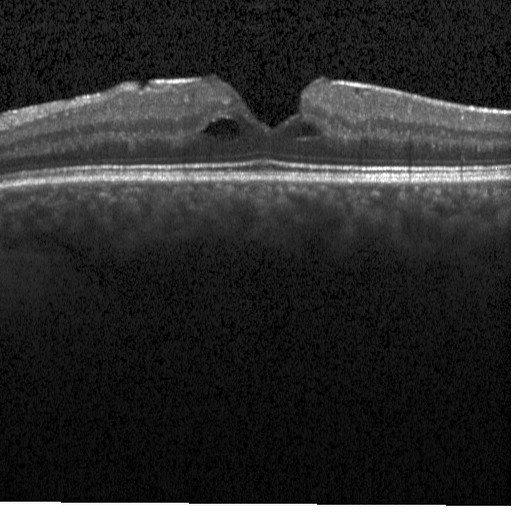

Retinal OCT cross-section showing DME.